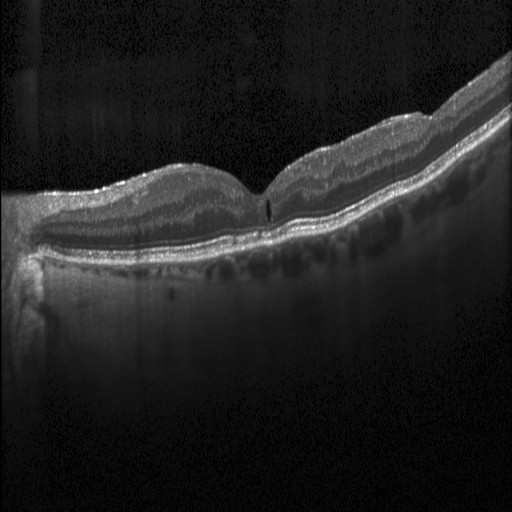 Retinal OCT cross-section · through the macula · SD-OCT — Diabetic macular edema.